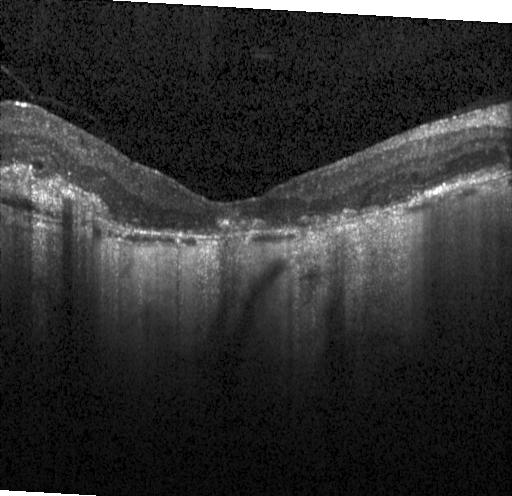 Heidelberg Spectralis OCT system, retinal OCT cross-section, spectral-domain OCT, macular scan. Choroidal neovascularization.